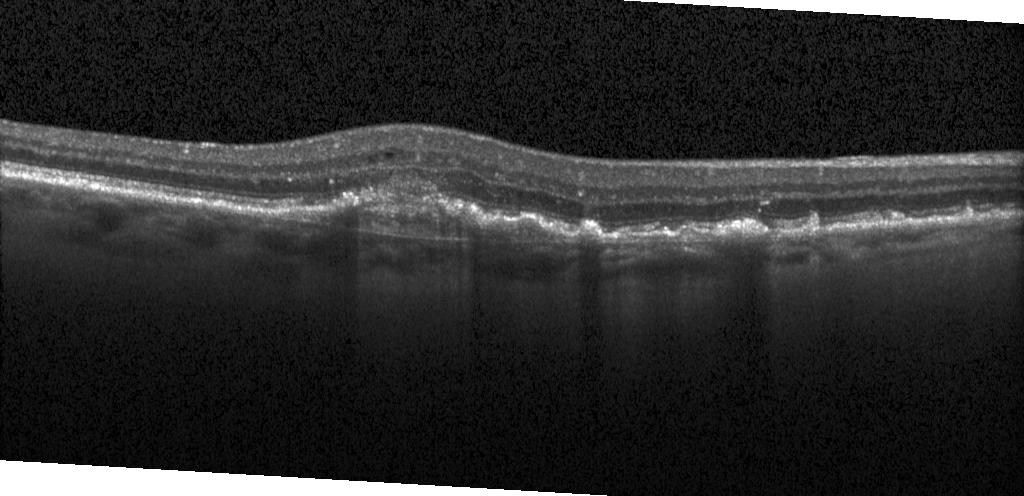
Assessment: choroidal neovascularization.